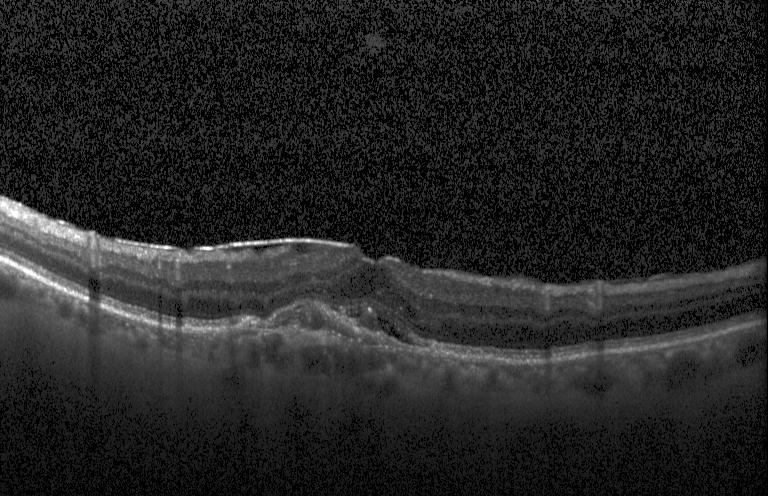
Retinal OCT cross-section. Finding: CNV.